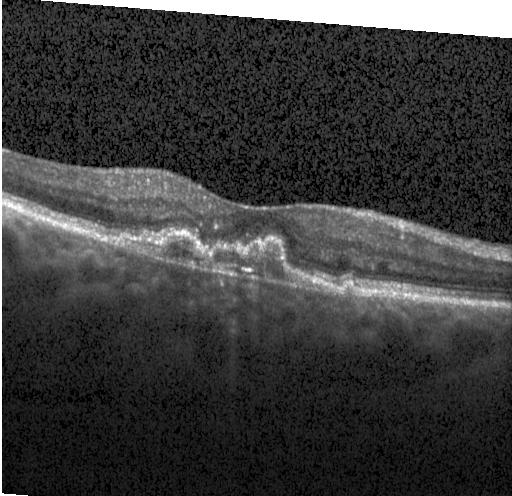
Retinal OCT cross-section showing a choroidal neovascular membrane.